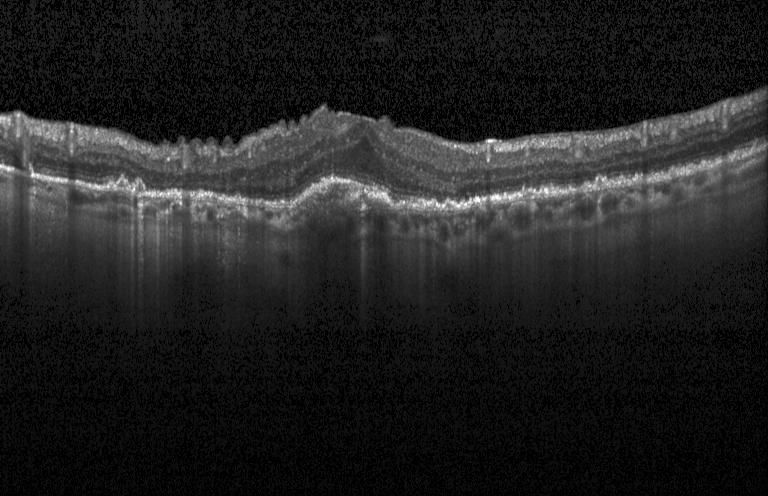
Retinal OCT B-scan. SD-OCT.
This B-scan demonstrates CNV.